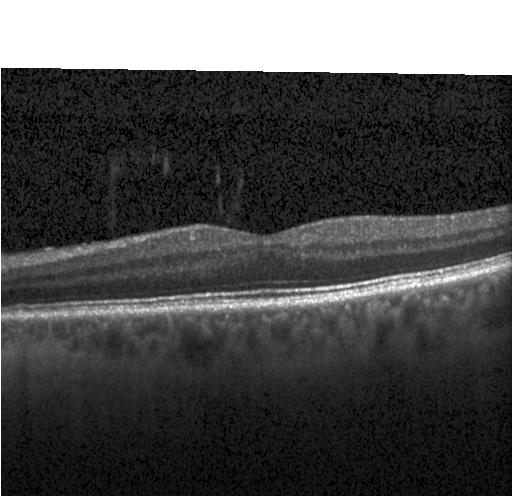

Optical coherence tomography B-scan. Finding: no evidence of CNV, DME, or drusen.